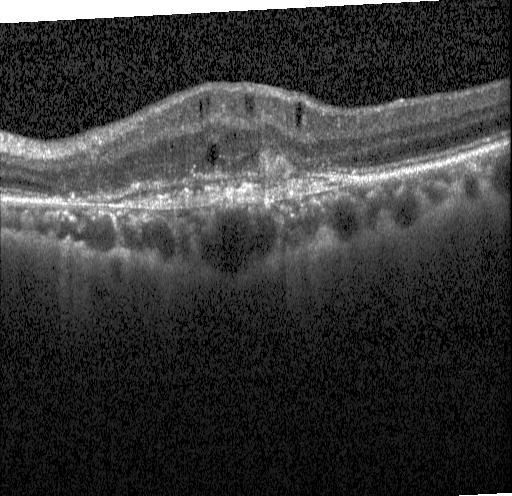

Spectral-domain OCT · Heidelberg Spectralis OCT system · OCT B-scan — Assessment: a choroidal neovascular membrane.